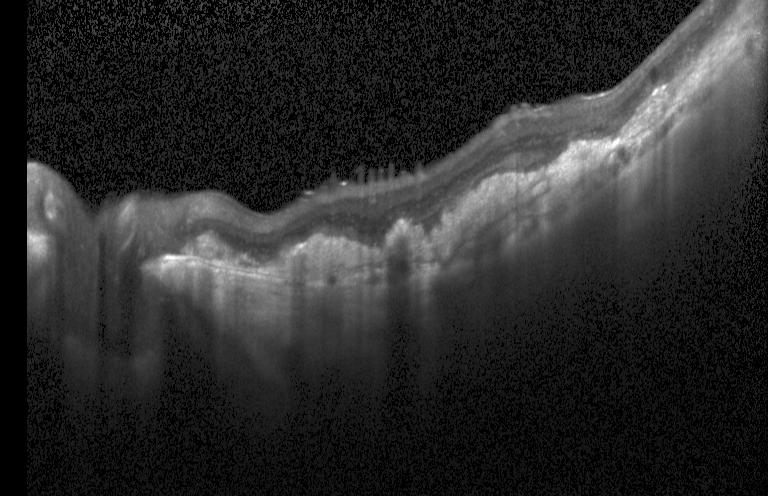

Optical coherence tomography B-scan. Spectral-domain optical coherence tomography. Acquired on a Heidelberg Spectralis.
The scan shows a choroidal neovascular membrane.